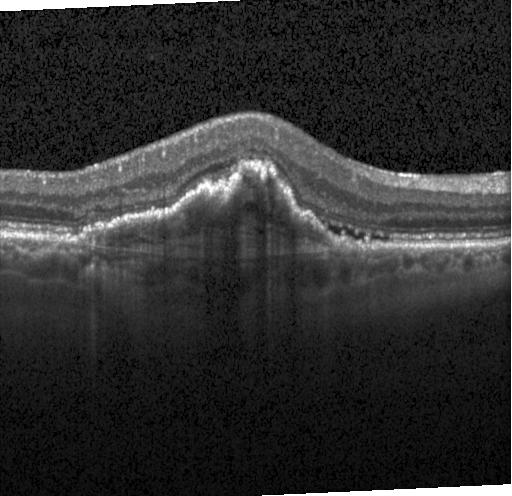

Heidelberg Spectralis OCT system, optical coherence tomography scan.
OCT finding: choroidal neovascularization.